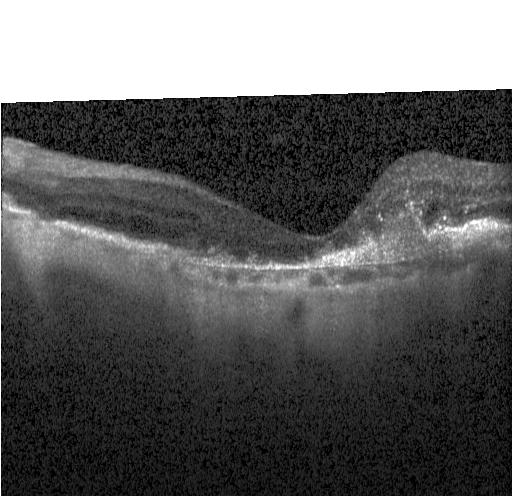

Centered on the fovea, Heidelberg Spectralis OCT system, optical coherence tomography B-scan — Impression: choroidal neovascularization (CNV).